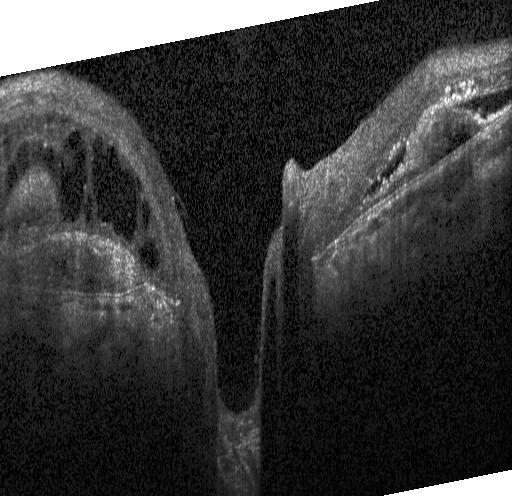 Fovea-centered. Spectral-domain OCT. Heidelberg Spectralis OCT system. Optical coherence tomography B-scan — Dx: a choroidal neovascular membrane.